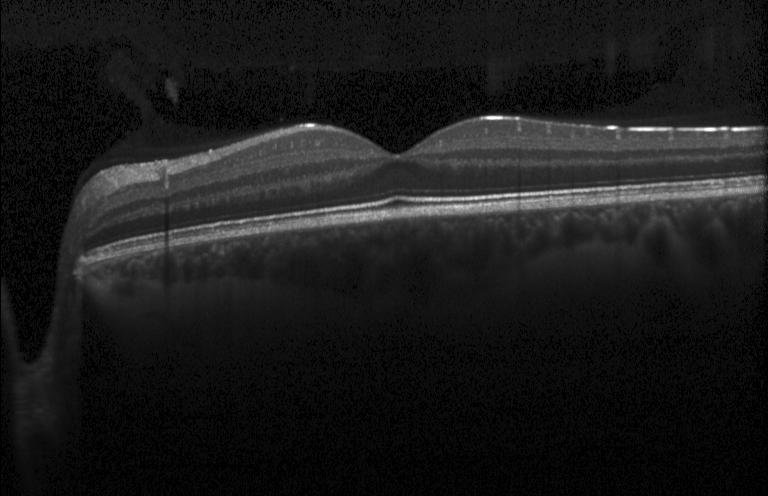

Retinal OCT B-scan; spectral-domain OCT; acquired on a Heidelberg Spectralis
Impression: no choroidal neovascularization, no diabetic macular edema, and no drusen.